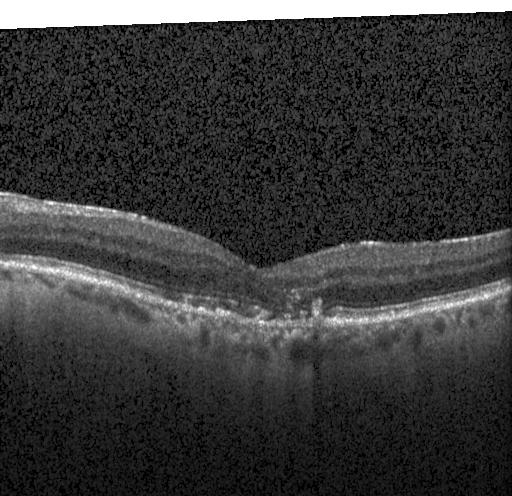
Finding: CNV.